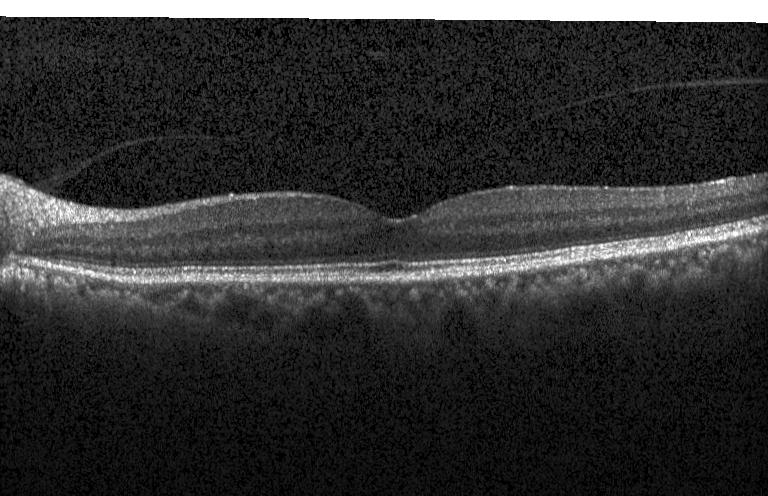

Macular OCT: no choroidal neovascularization, diabetic macular edema, or drusen.